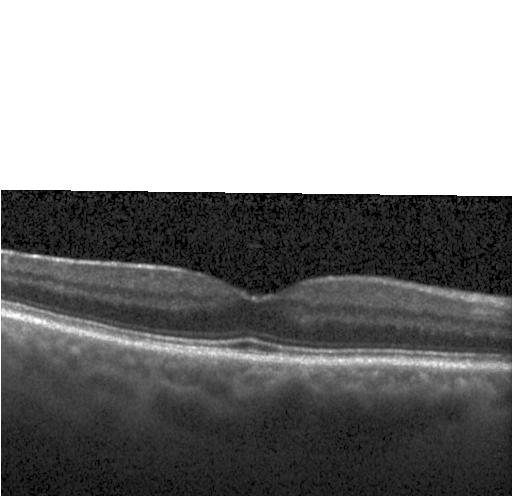

Optical coherence tomography scan, through the macula
Diagnosis: no choroidal neovascularization, diabetic macular edema, or drusen.